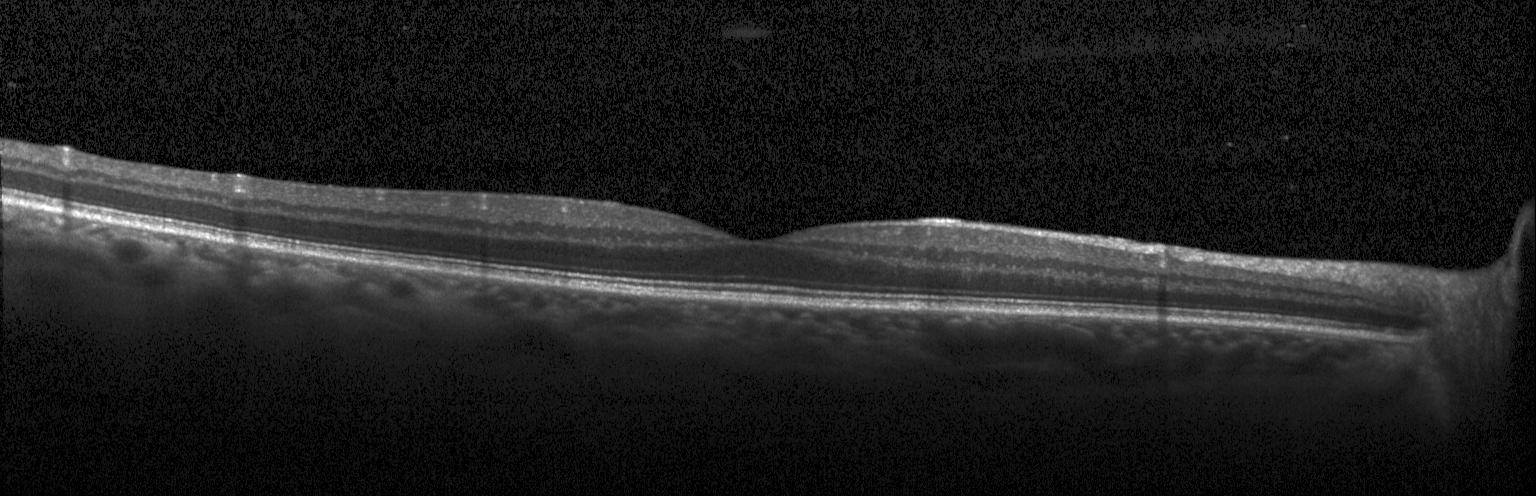
Impression: no evidence of choroidal neovascularization, diabetic macular edema, or drusen.